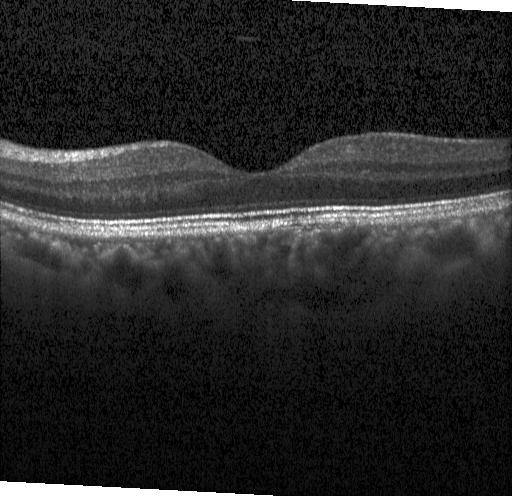
Fovea-centered, spectral-domain optical coherence tomography, Heidelberg Spectralis OCT system, OCT B-scan.
The scan shows no evidence of choroidal neovascularization, diabetic macular edema, or drusen.